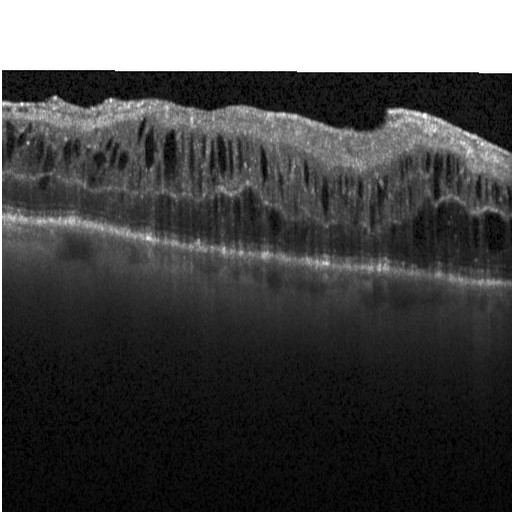
Spectral-domain OCT · retinal OCT cross-section · acquired on a Heidelberg Spectralis · centered on the fovea.
Assessment: DME.